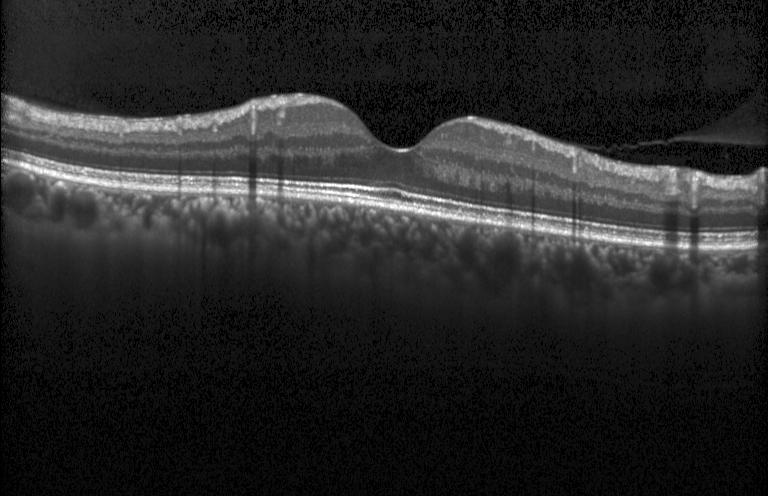 Through the macula; OCT line scan; instrument: Heidelberg Spectralis.
This B-scan demonstrates no CNV, DME, or drusen.